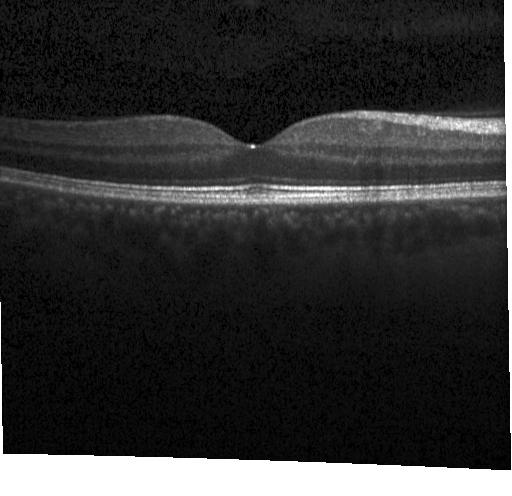

Impression: no evidence of choroidal neovascularization, diabetic macular edema, or drusen.